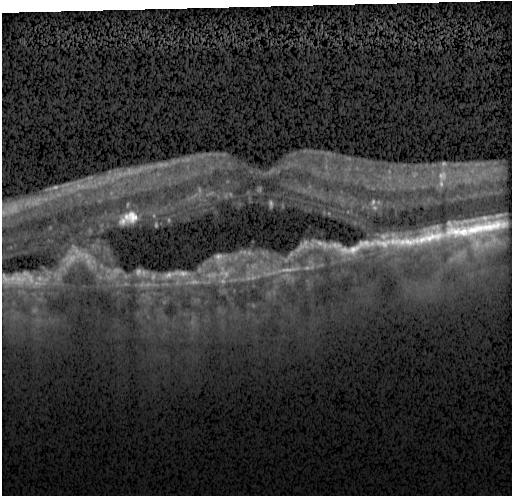

Spectral-domain OCT · fovea-centered · retinal OCT B-scan · instrument: Heidelberg Spectralis
Assessment: choroidal neovascularization.